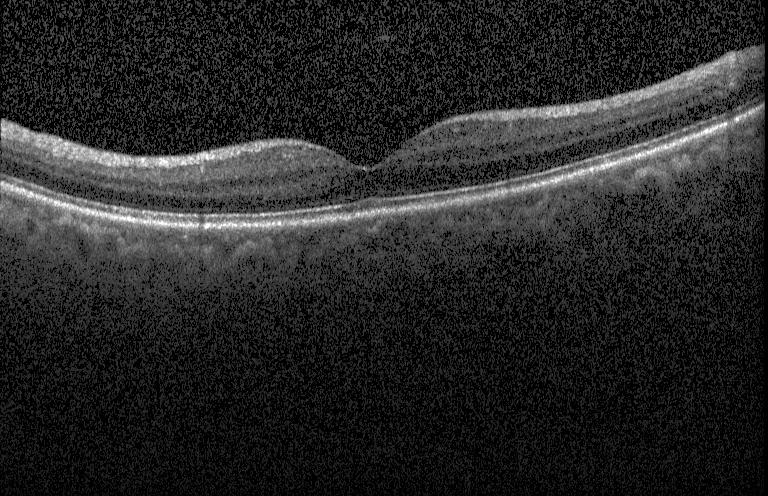 Heidelberg Spectralis, centered on the fovea, spectral-domain OCT, OCT B-scan
The scan shows no choroidal neovascularization, diabetic macular edema, or drusen.